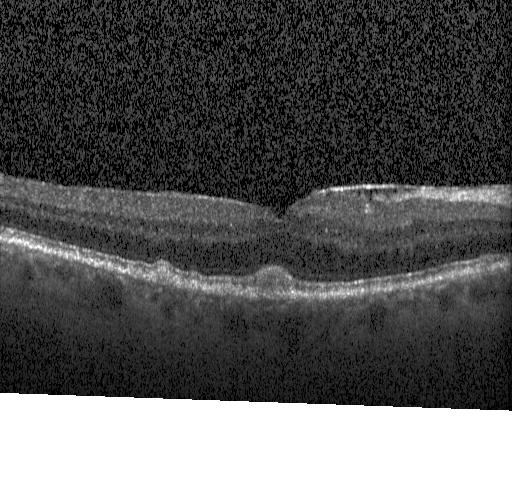
Impression: sub-RPE drusenoid deposits.